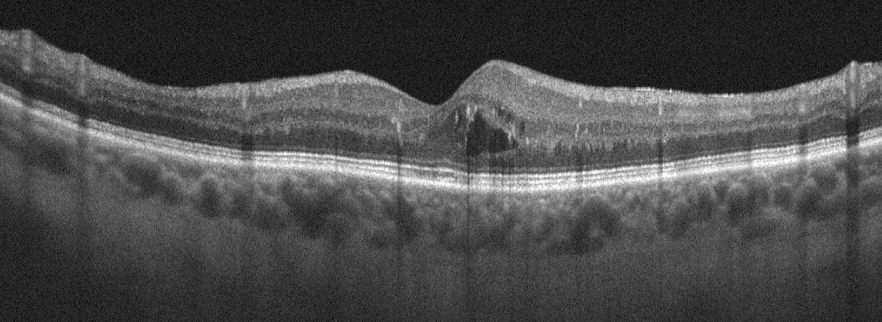
OCT line scan, macular scan — Diagnosis: diabetic macular edema (DME).